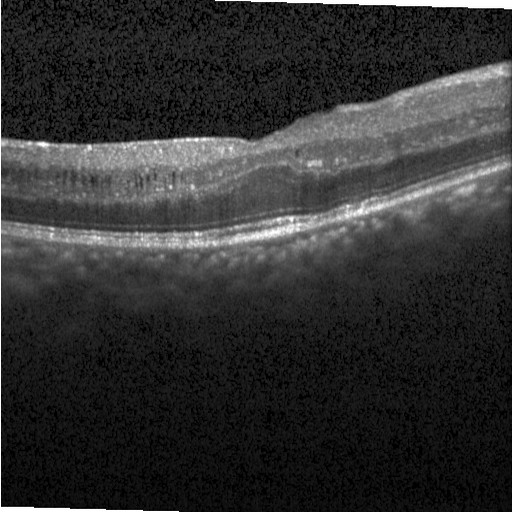
Finding: DME.